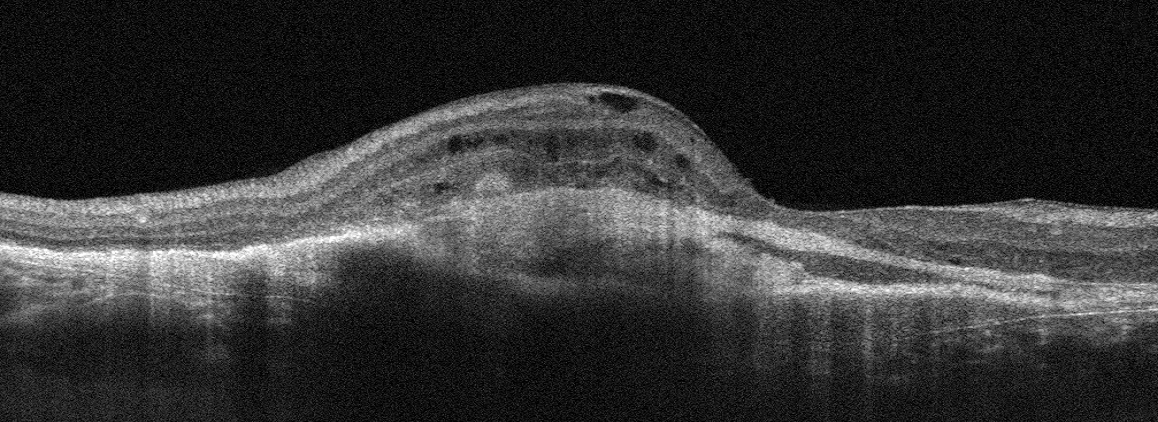
OCT B-scan · right eye
The scan shows AMD.